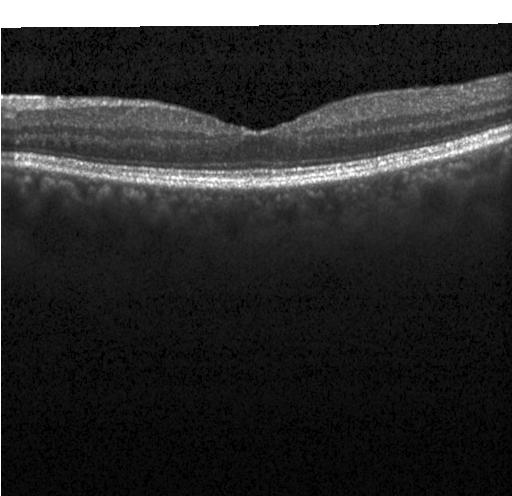
Retinal OCT cross-section showing no evidence of CNV, DME, or drusen.